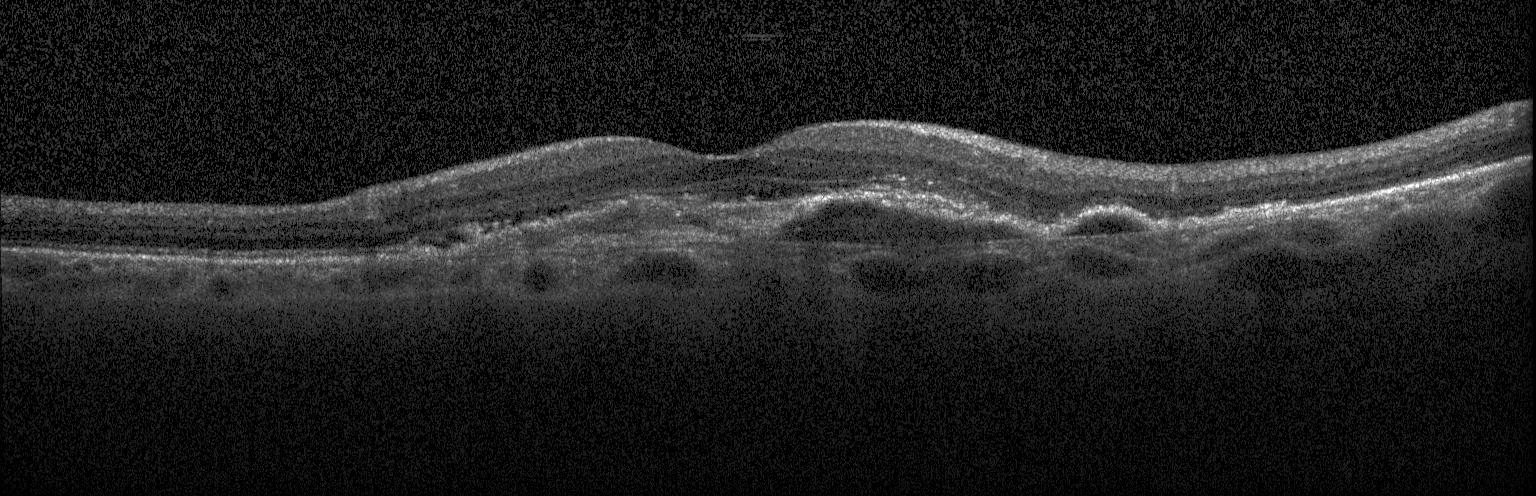

Centered on the fovea, optical coherence tomography scan — This B-scan demonstrates choroidal neovascularization.